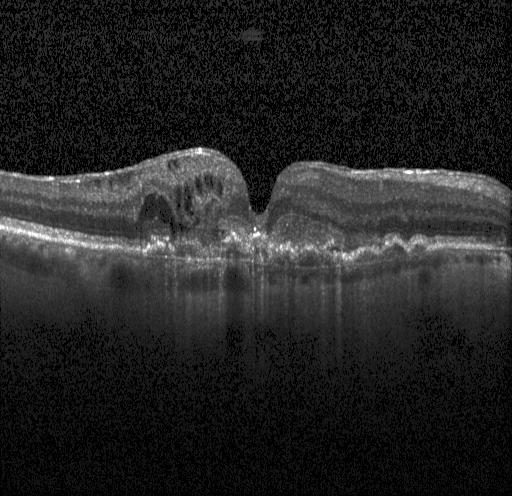

Instrument: Heidelberg Spectralis, SD-OCT, optical coherence tomography B-scan, macular scan
Dx: choroidal neovascularization.